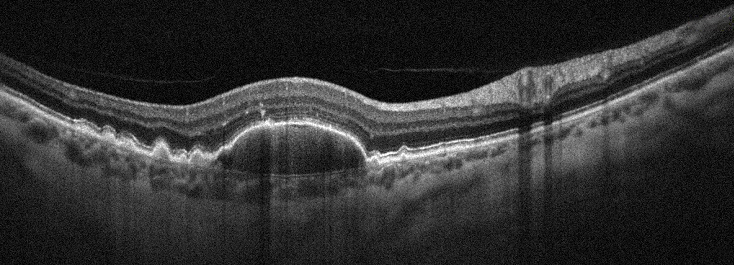
Optovue Avanti RTVue XR · optical coherence tomography B-scan — OCT finding: age-related macular degeneration.